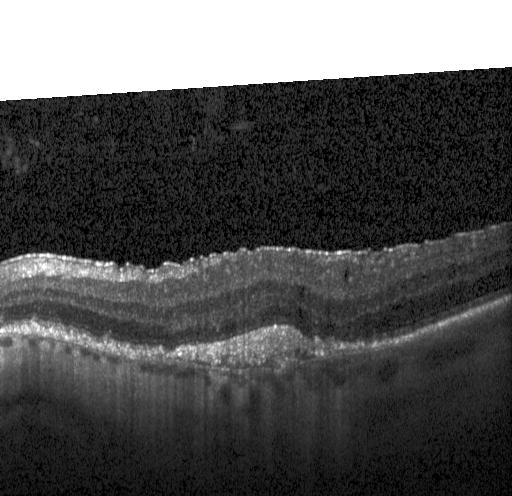

Dx: choroidal neovascularization.